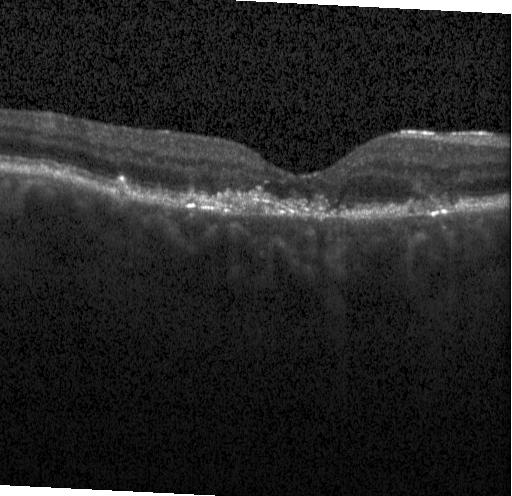
OCT line scan.
Diagnosis: CNV.